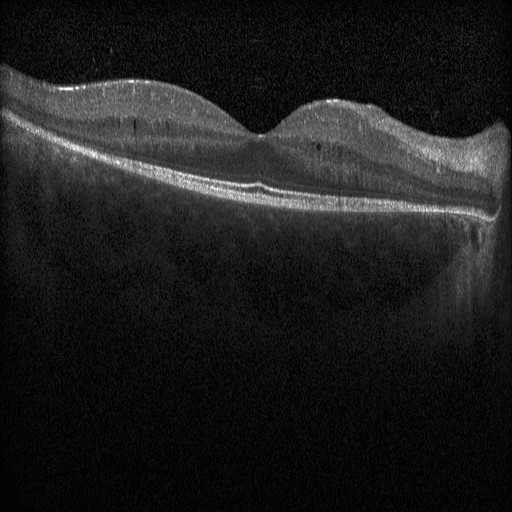

Diagnosis: DME.